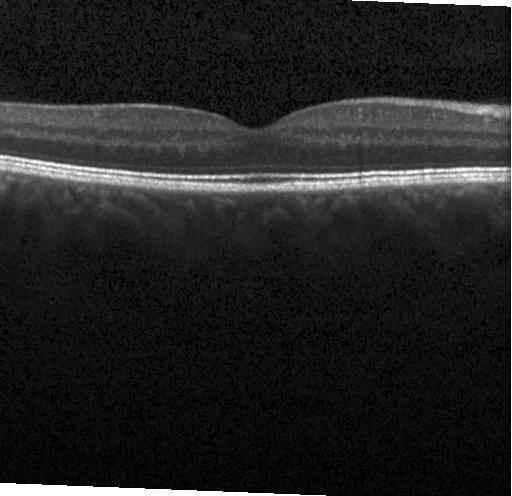
Macular OCT demonstrating no evidence of choroidal neovascularization, diabetic macular edema, or drusen.